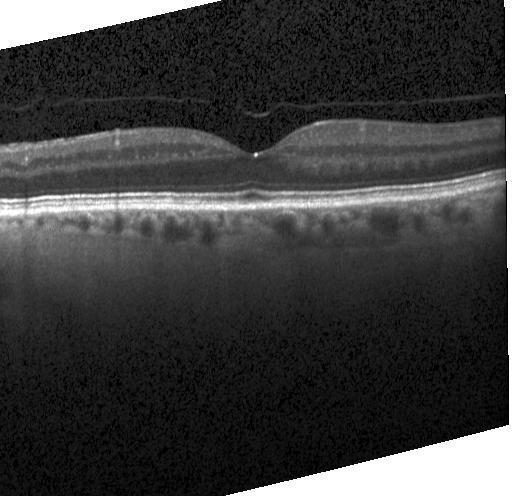
Heidelberg Spectralis; retinal OCT B-scan.
Finding: no choroidal neovascularization, diabetic macular edema, or drusen.